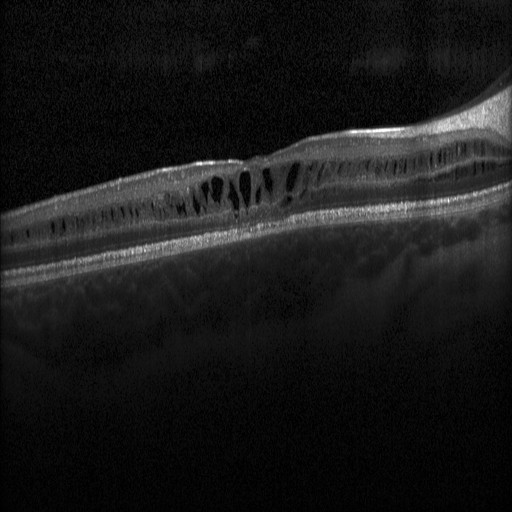 OCT line scan, through the macula. Finding: diabetic macular edema.